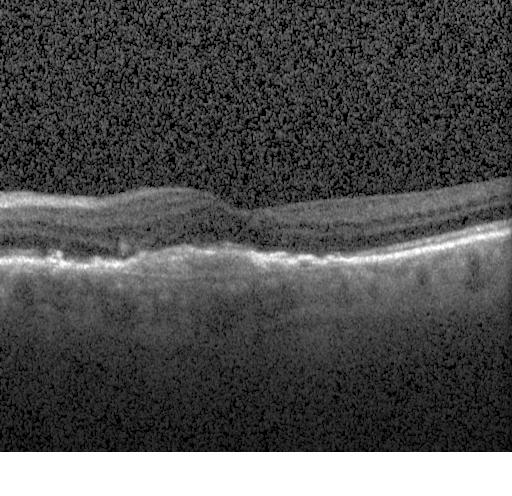
Retinal OCT B-scan · Heidelberg Spectralis OCT system · through the macula.
Finding: CNV.